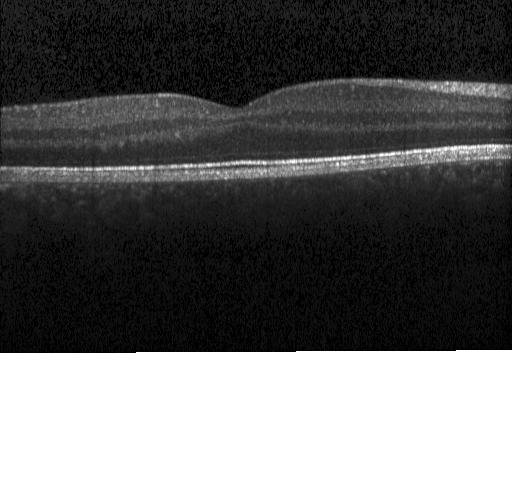
Spectral-domain OCT, horizontal scan through the fovea, instrument: Heidelberg Spectralis, retinal OCT B-scan. Dx: no CNV, no DME, and no drusen.